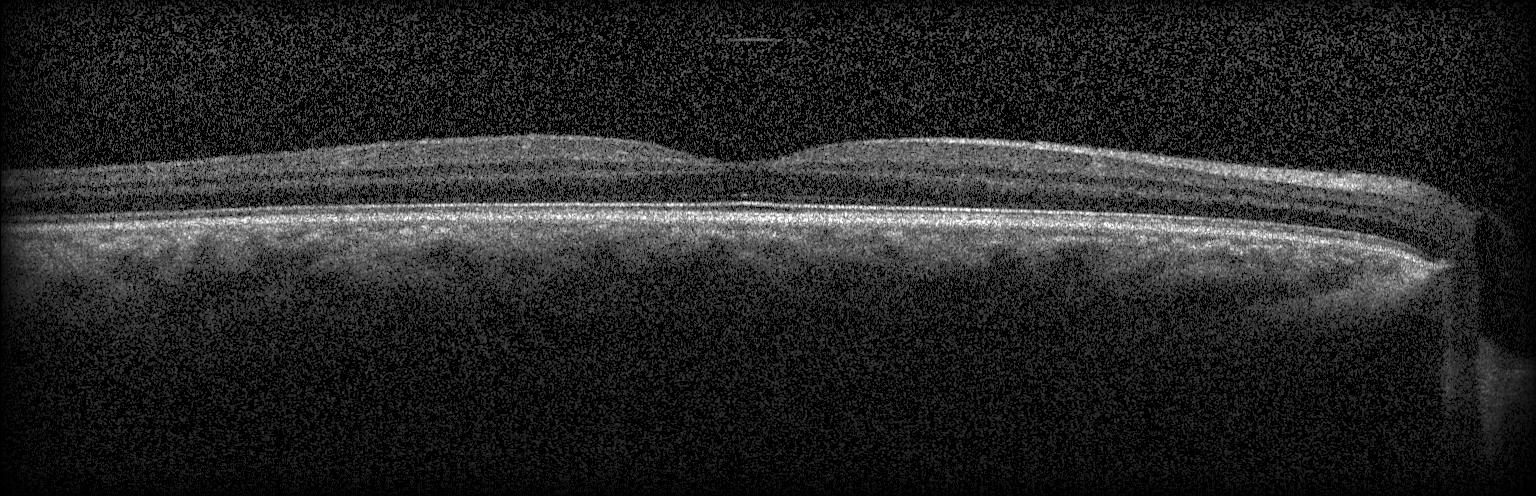 SD-OCT · Heidelberg Spectralis · optical coherence tomography B-scan. Macular OCT: neither choroidal neovascularization, diabetic macular edema, nor drusen.